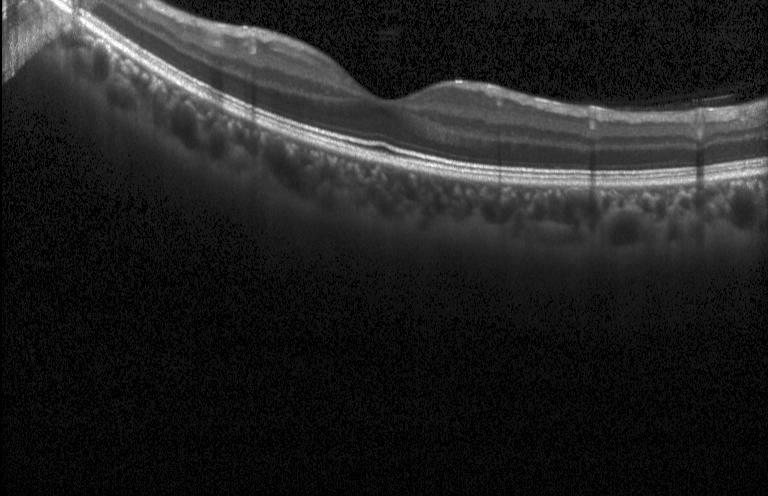 No evidence of CNV, DME, or drusen.